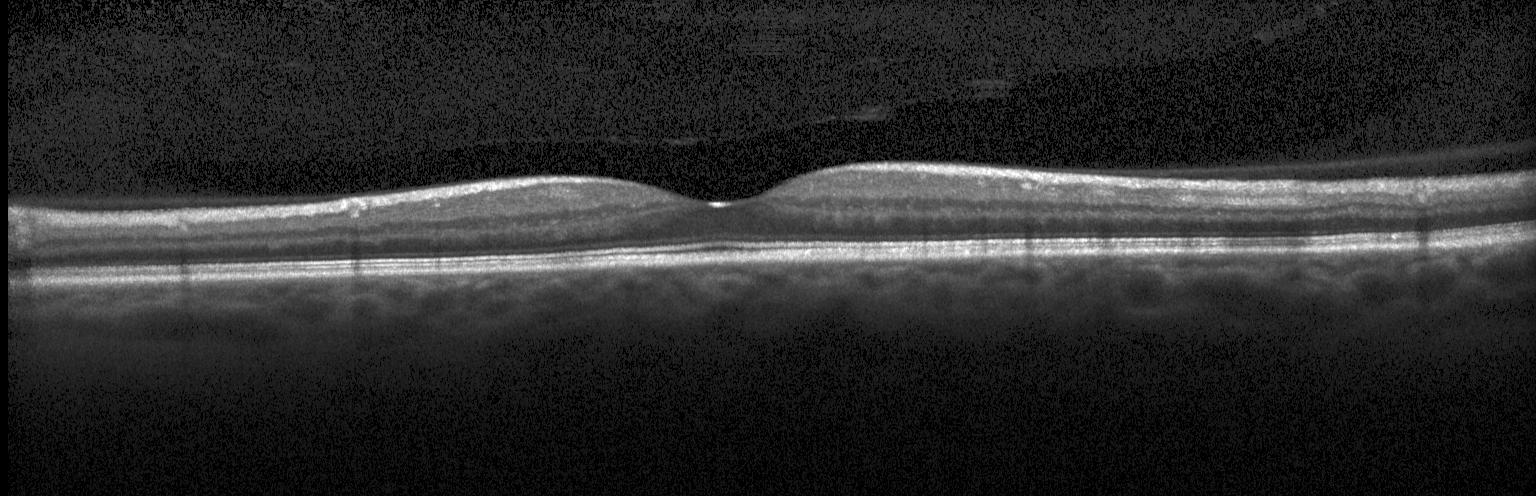

Spectral-domain OCT, Heidelberg Spectralis, retinal OCT cross-section.
Neither choroidal neovascularization, diabetic macular edema, nor drusen.